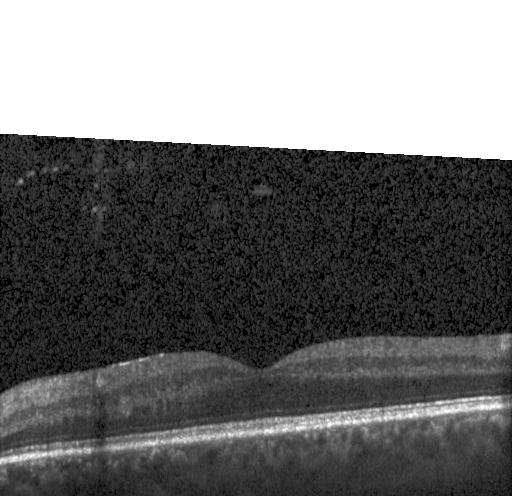
OCT B-scan — Neither choroidal neovascularization, diabetic macular edema, nor drusen.